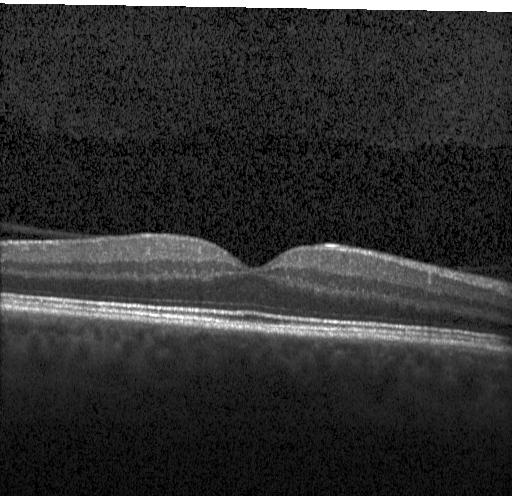
Neither choroidal neovascularization, diabetic macular edema, nor drusen.